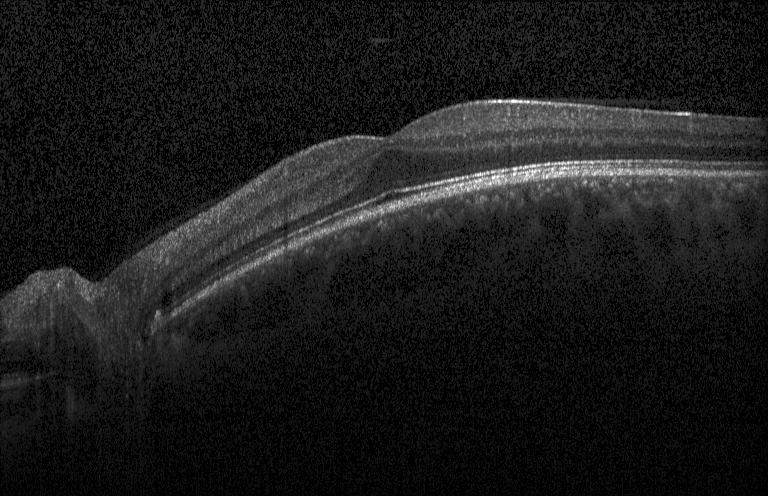 Through the macula; acquired on a Heidelberg Spectralis; optical coherence tomography scan; spectral-domain optical coherence tomography. Assessment: neither choroidal neovascularization, diabetic macular edema, nor drusen.